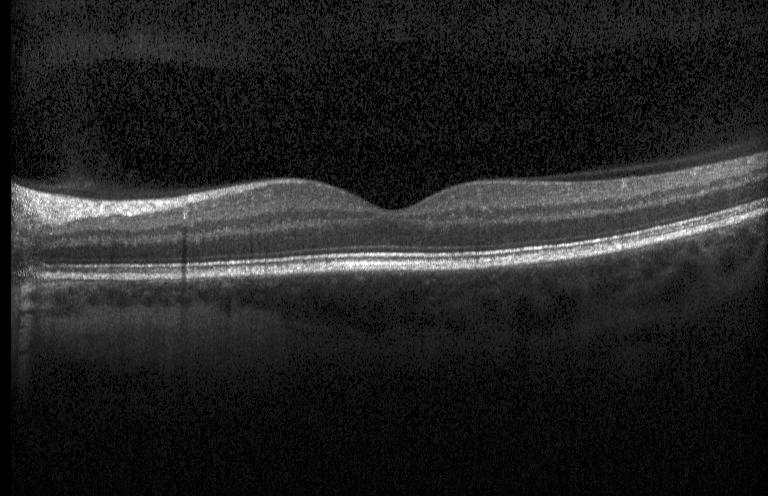

Neither choroidal neovascularization, diabetic macular edema, nor drusen.